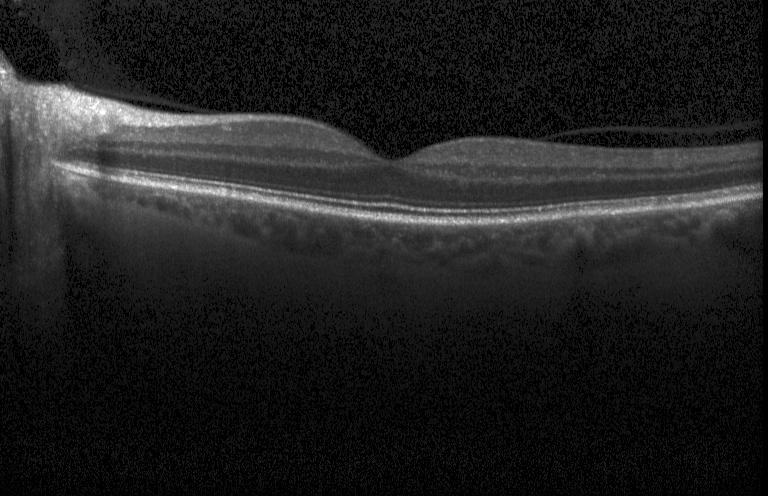 SD-OCT. OCT B-scan. Acquired on a Heidelberg Spectralis. Macular scan — Diagnosis: no choroidal neovascularization, diabetic macular edema, or drusen.